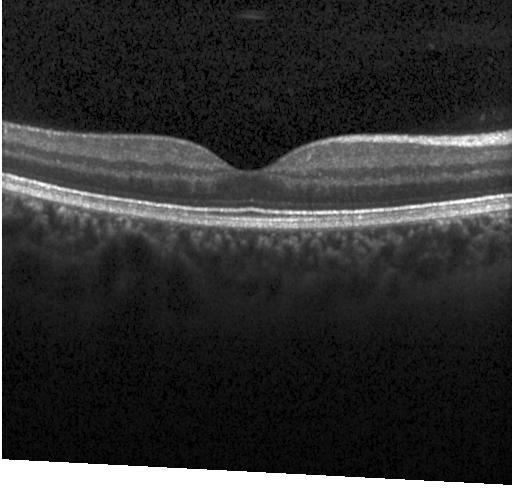 Optical coherence tomography B-scan
This B-scan demonstrates no choroidal neovascularization, diabetic macular edema, or drusen.